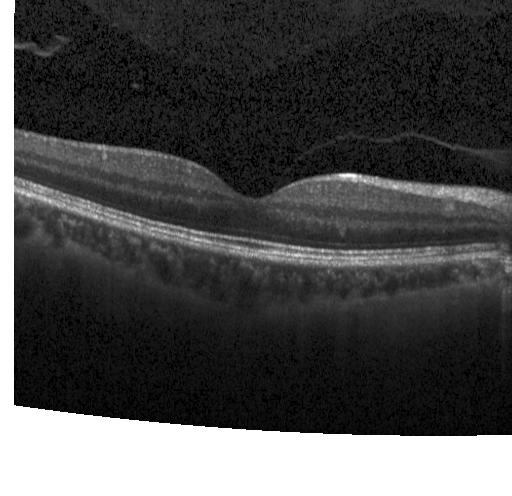 Retinal OCT B-scan, spectral-domain optical coherence tomography. Impression: no CNV, no DME, and no drusen.